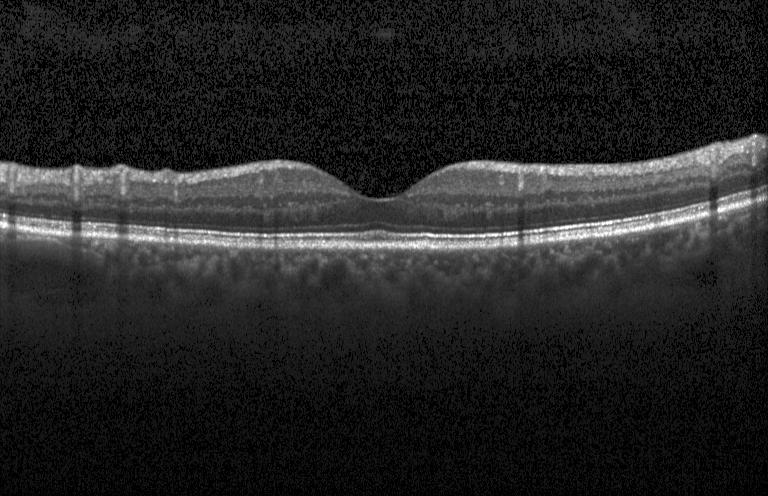

No evidence of choroidal neovascularization, diabetic macular edema, or drusen.